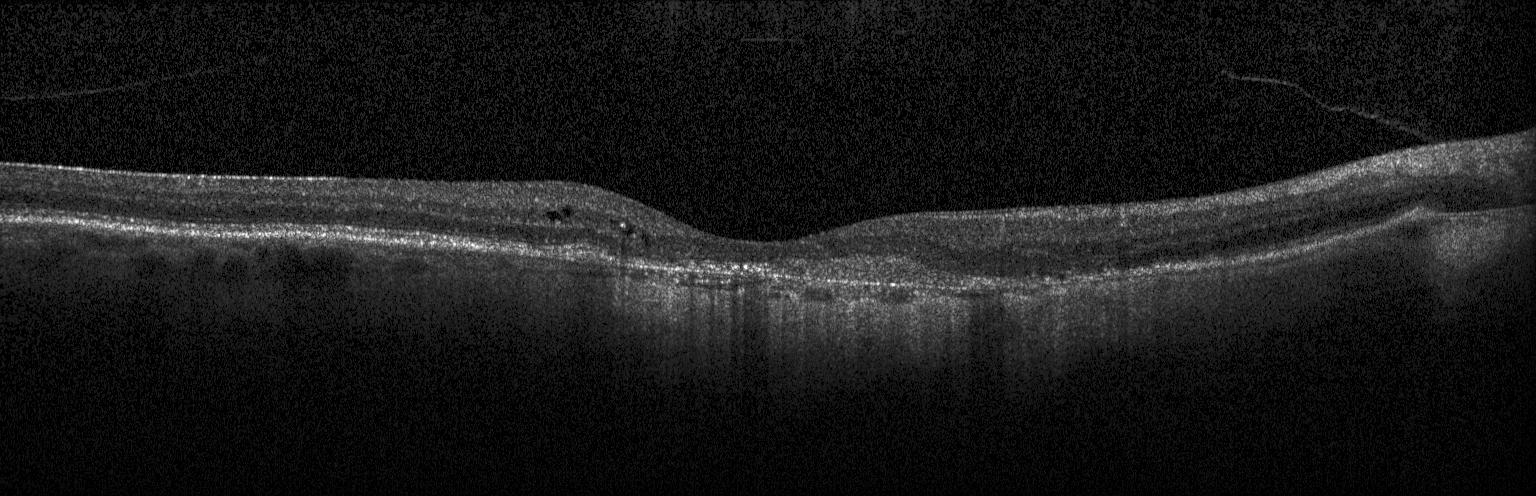 Retinal OCT B-scan. Diagnosis: a choroidal neovascular membrane.